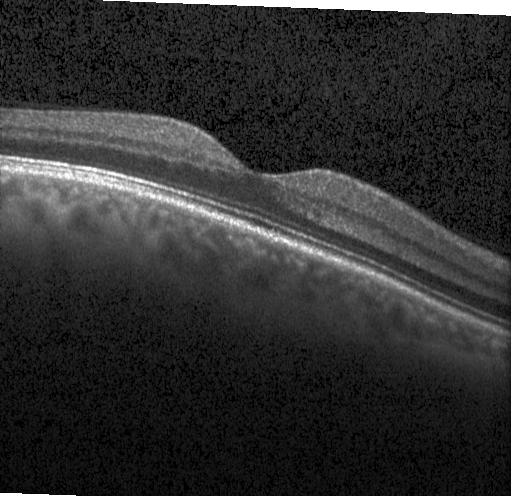 Spectral-domain OCT, centered on the fovea, OCT line scan. Macular OCT: no evidence of CNV, DME, or drusen.